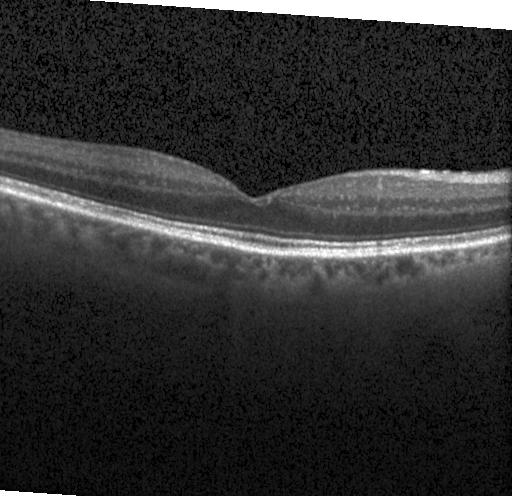

No CNV, no DME, and no drusen.